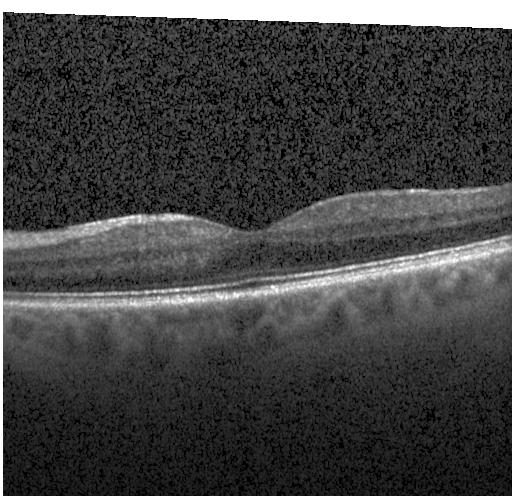
The scan shows no evidence of choroidal neovascularization, diabetic macular edema, or drusen.